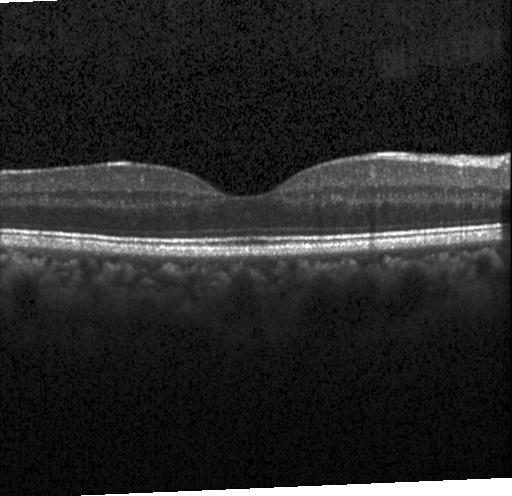
Impression: neither CNV, DME, nor drusen.